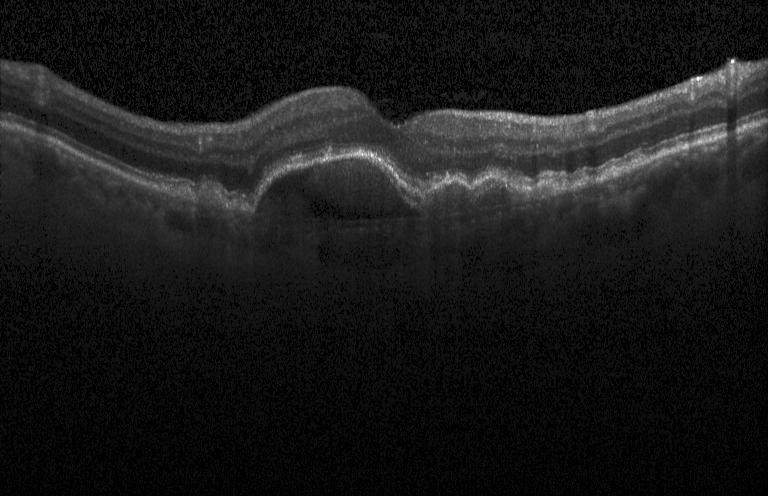

Optical coherence tomography B-scan · fovea-centered.
Diagnosis: sub-RPE drusenoid deposits.